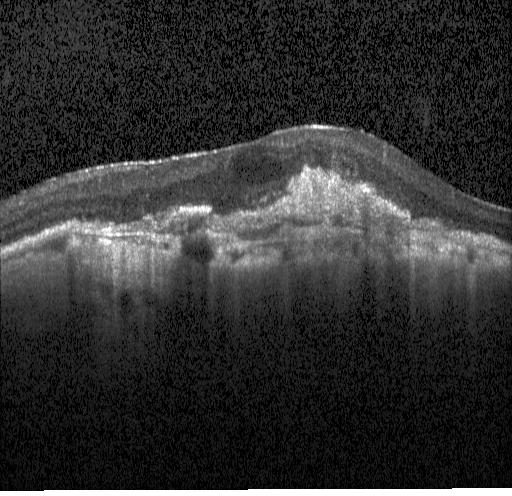
Spectral-domain optical coherence tomography · centered on the fovea · optical coherence tomography scan. Diagnosis: CNV.